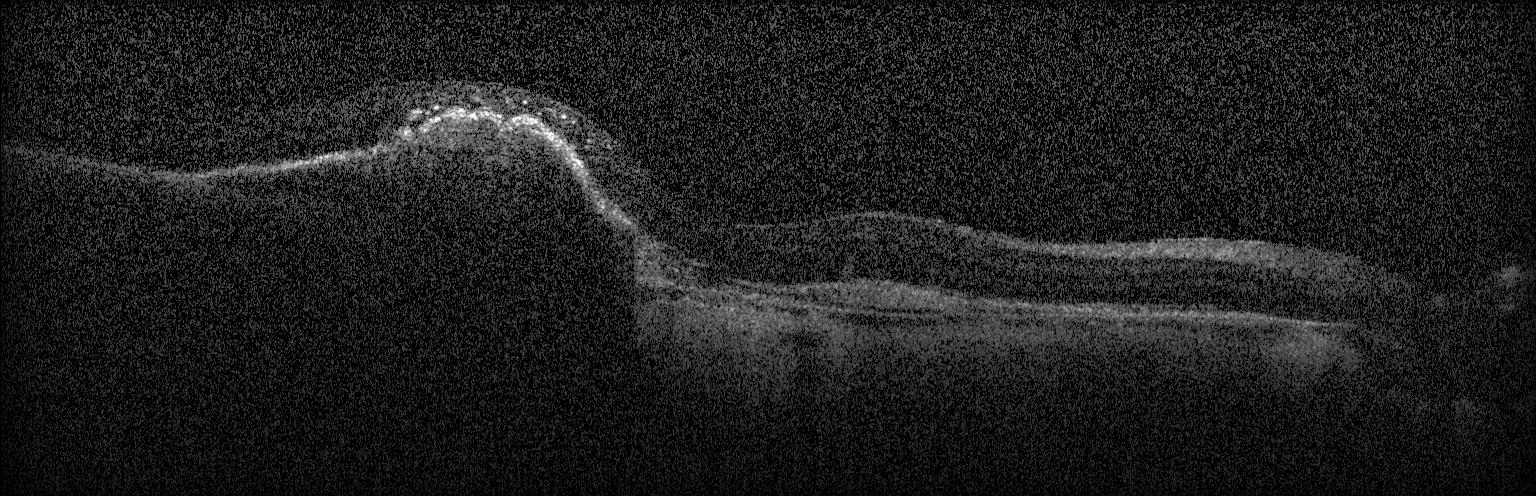
OCT finding: a choroidal neovascular membrane.